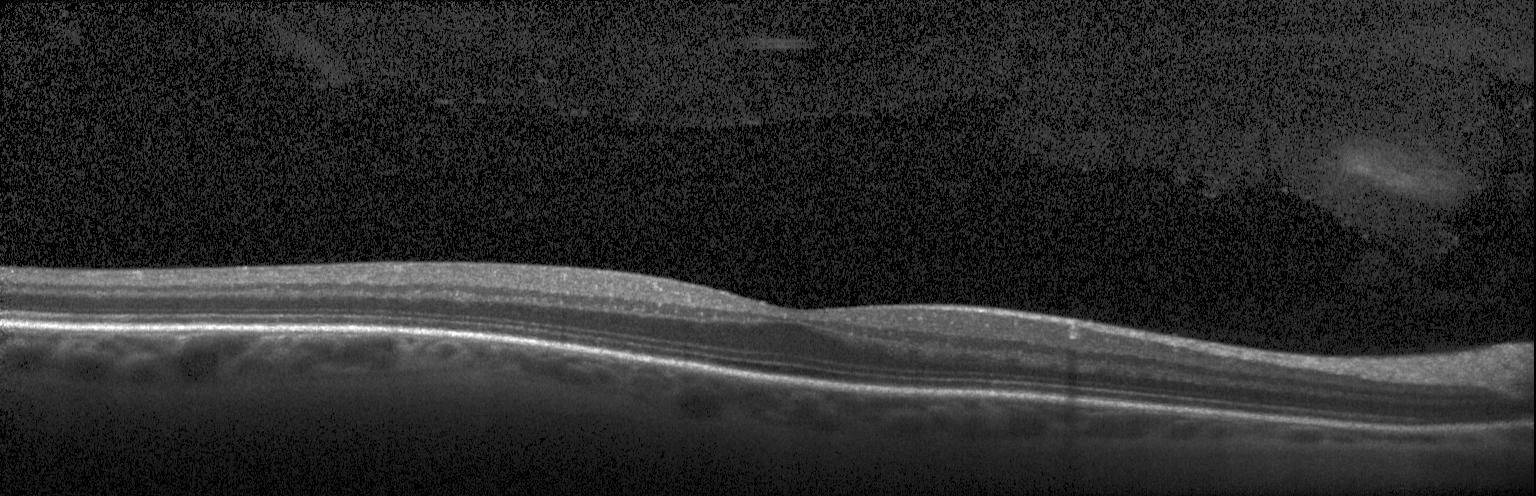 Impression: no evidence of CNV, DME, or drusen.